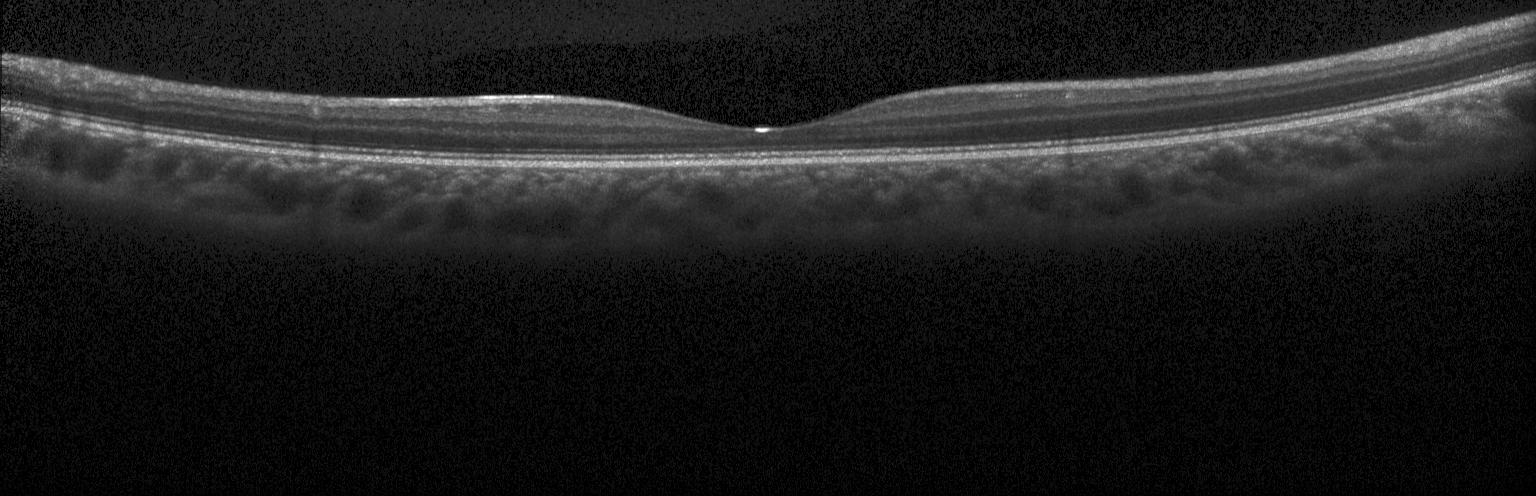
OCT finding: neither CNV, DME, nor drusen.